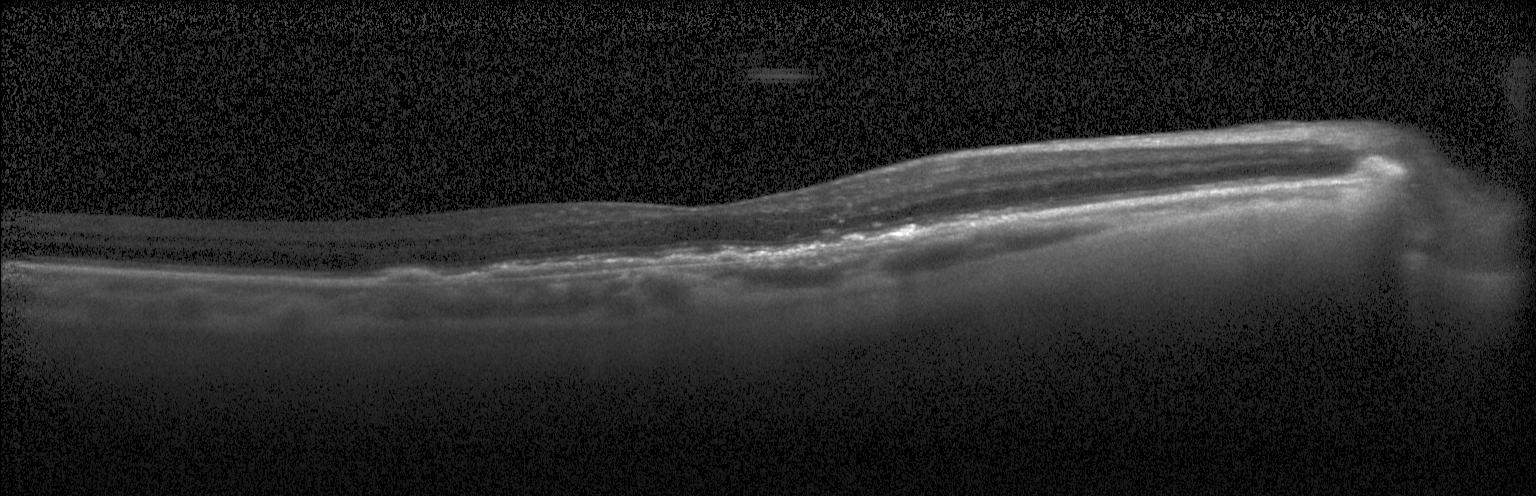 OCT B-scan showing choroidal neovascularization (CNV).